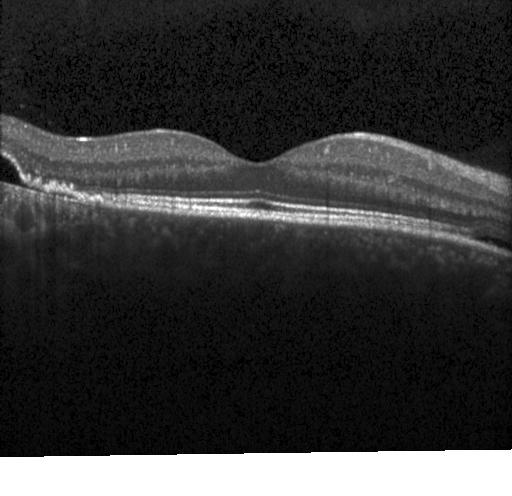

Macular OCT: CNV.